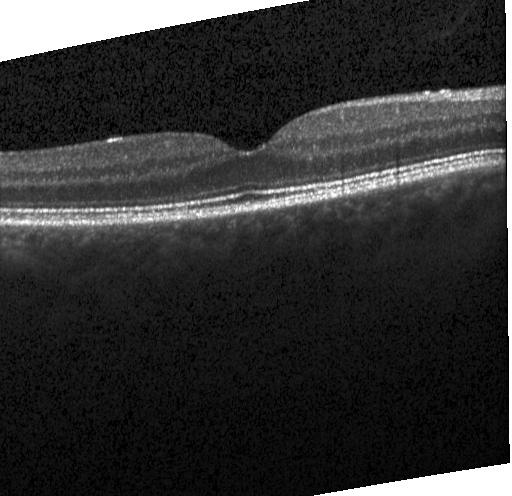 Optical coherence tomography scan. Centered on the fovea. Heidelberg Spectralis OCT system
Assessment: neither choroidal neovascularization, diabetic macular edema, nor drusen.